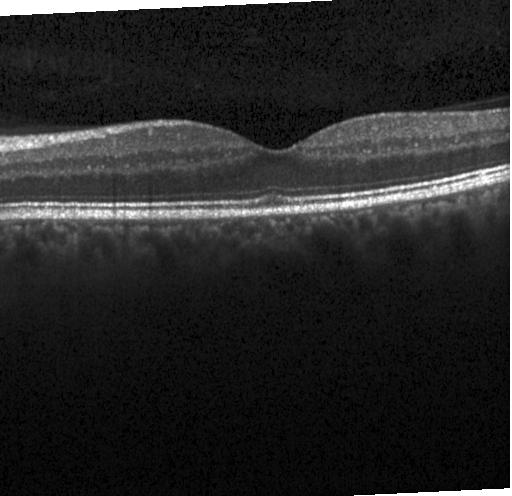 Diagnosis: no CNV, DME, or drusen.